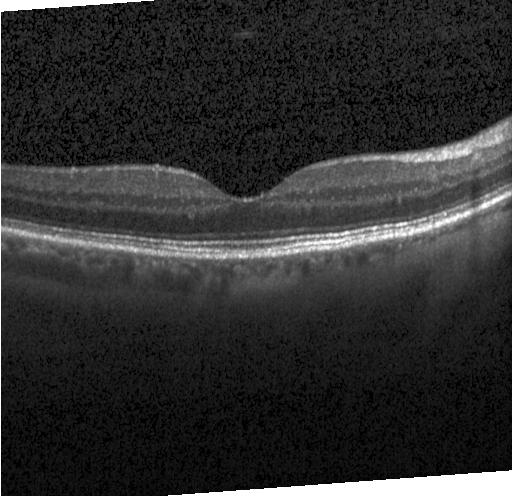
Optical coherence tomography scan. Diagnosis: no choroidal neovascularization, diabetic macular edema, or drusen.